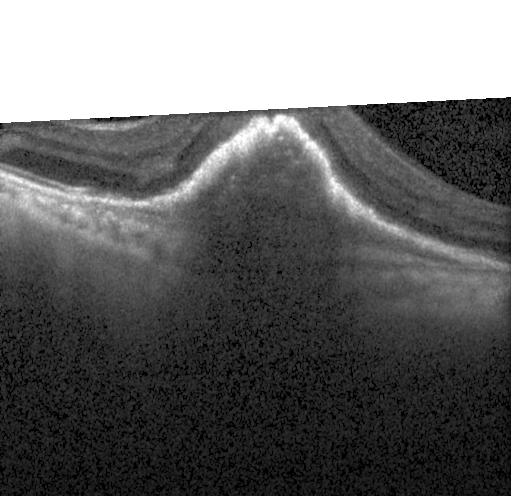

Diagnosis: a choroidal neovascular membrane.